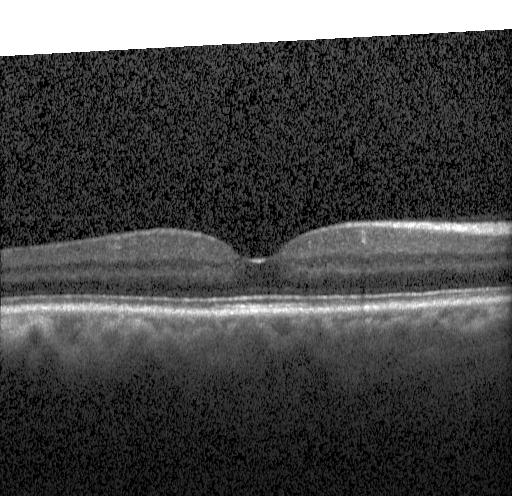

Spectral-domain OCT B-scan: no choroidal neovascularization, no diabetic macular edema, and no drusen.